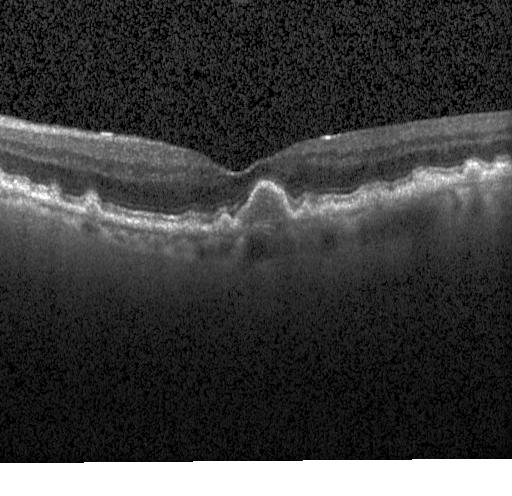 OCT scan showing sub-RPE drusenoid deposits.